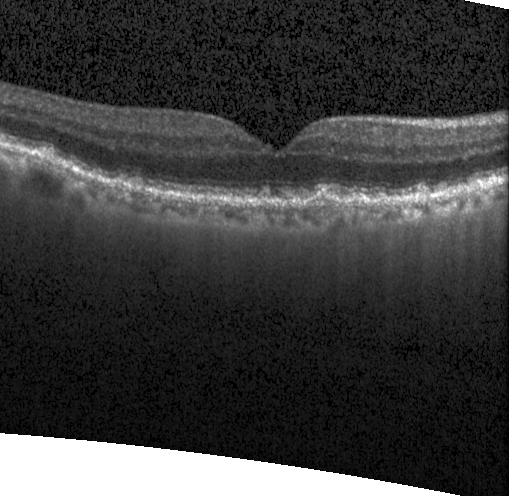

Spectral-domain OCT. Optical coherence tomography B-scan. OCT finding: drusen.